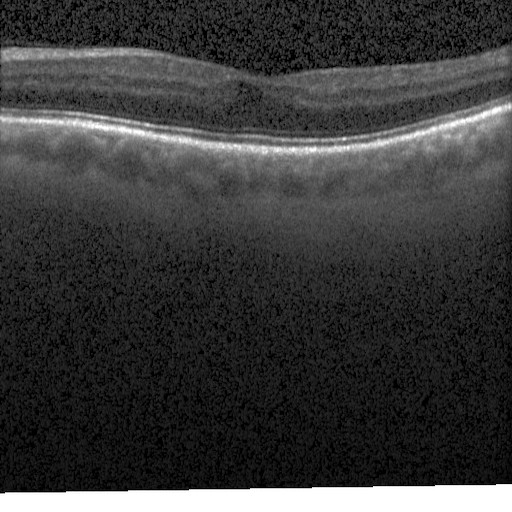
Spectral-domain OCT, fovea-centered, OCT line scan.
Dx: diabetic macular edema.